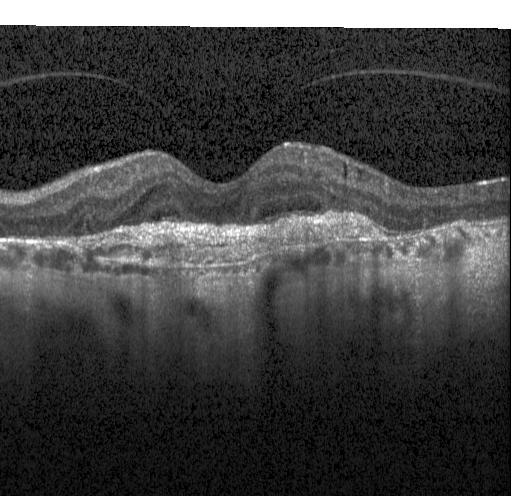 Heidelberg Spectralis, optical coherence tomography B-scan, horizontal scan through the fovea.
Impression: a choroidal neovascular membrane.